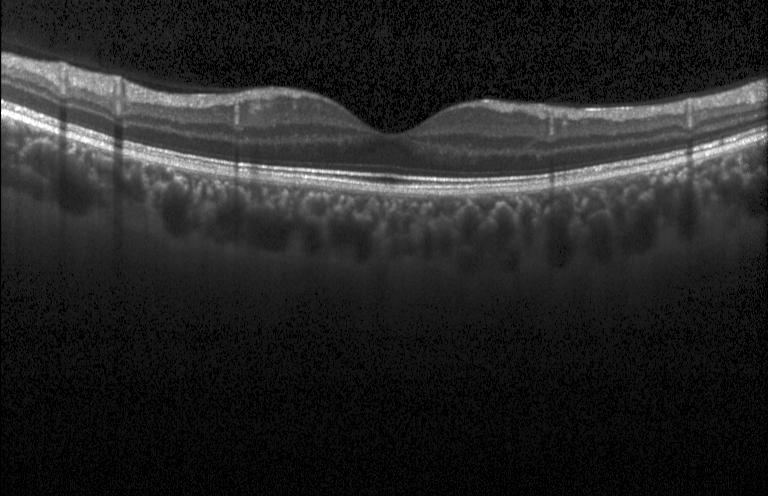

SD-OCT; acquired on a Heidelberg Spectralis; OCT line scan; horizontal scan through the fovea — Impression: no CNV, no DME, and no drusen.